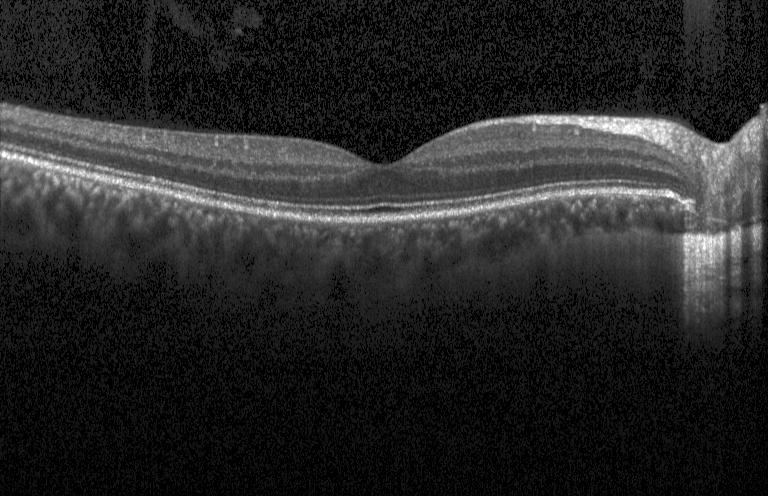

Spectral-domain OCT; instrument: Heidelberg Spectralis; retinal OCT B-scan; macular scan — No evidence of CNV, DME, or drusen.